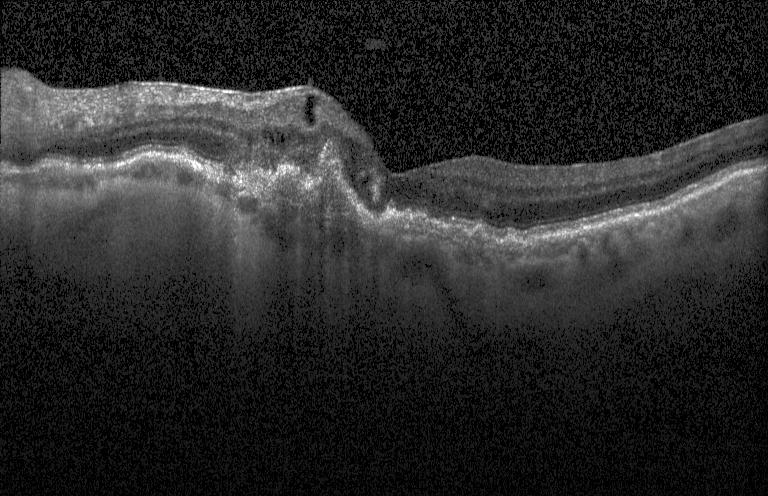
SD-OCT · optical coherence tomography B-scan · Heidelberg Spectralis · horizontal scan through the fovea
Dx: choroidal neovascularization.